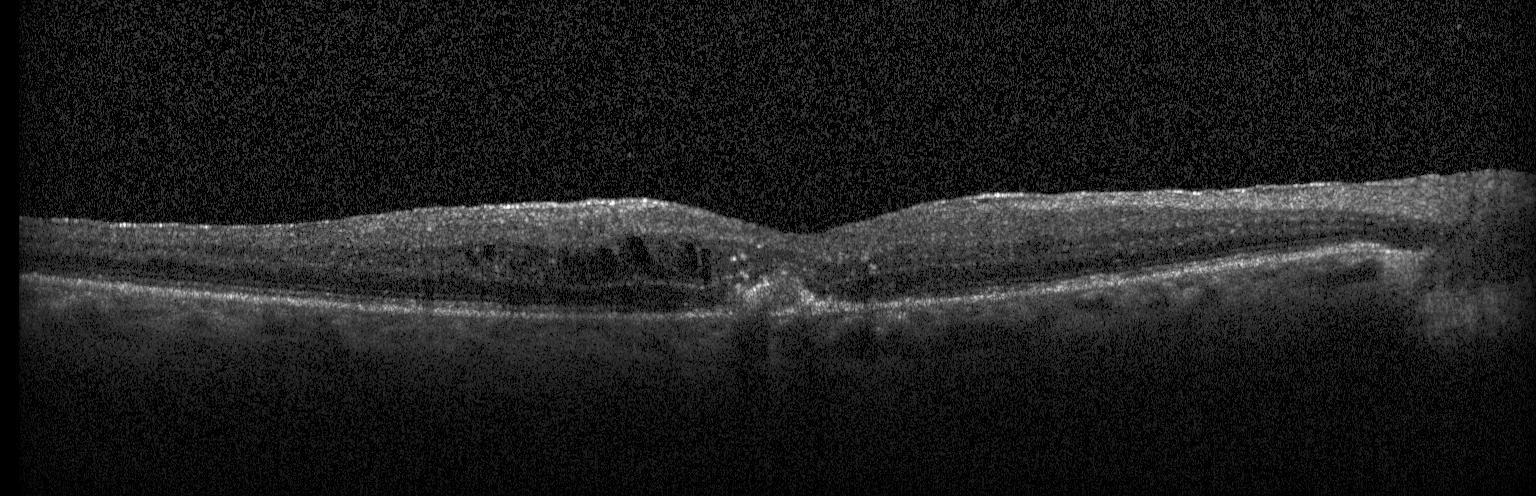
OCT line scan · spectral-domain OCT · through the macula — OCT finding: CNV.